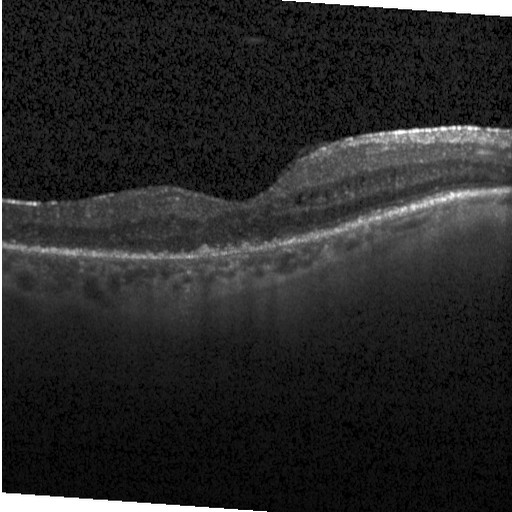

OCT line scan. Finding: diabetic macular edema (DME).